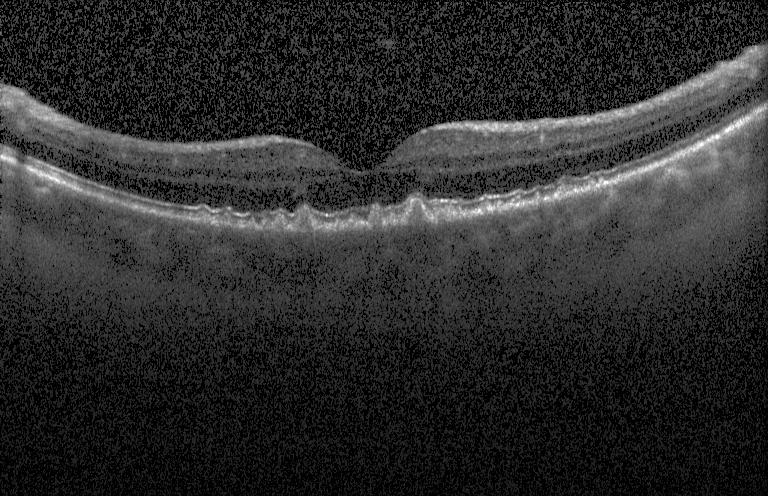 Spectral-domain OCT B-scan: sub-RPE drusenoid deposits.